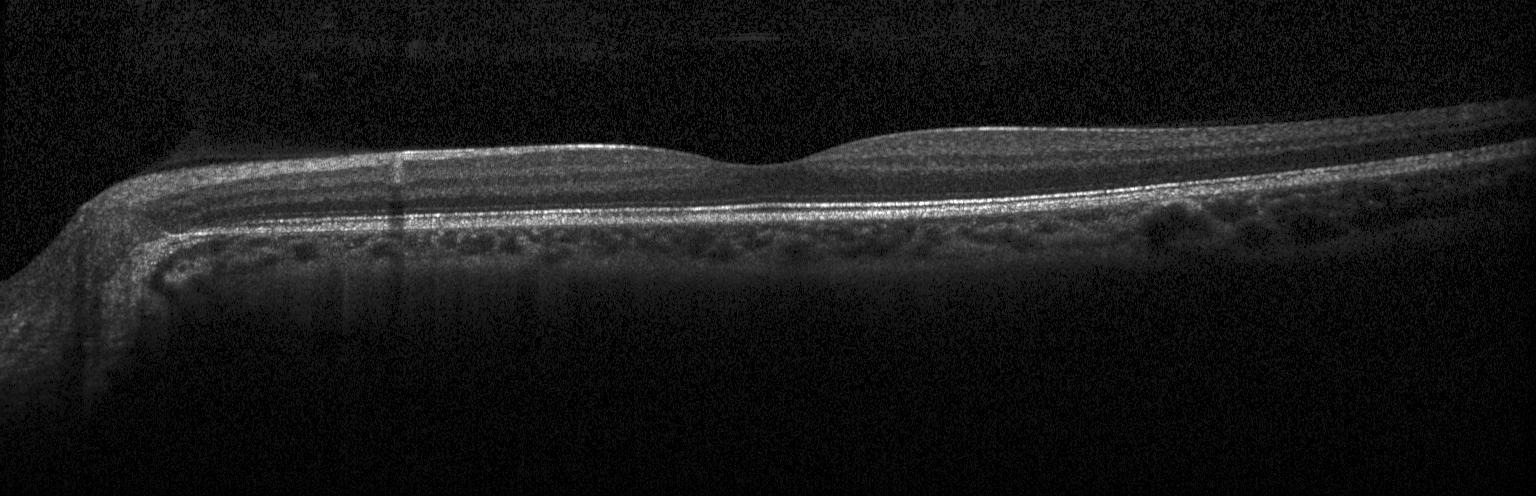
Centered on the fovea; instrument: Heidelberg Spectralis; optical coherence tomography B-scan; spectral-domain OCT. Impression: no choroidal neovascularization, no diabetic macular edema, and no drusen.